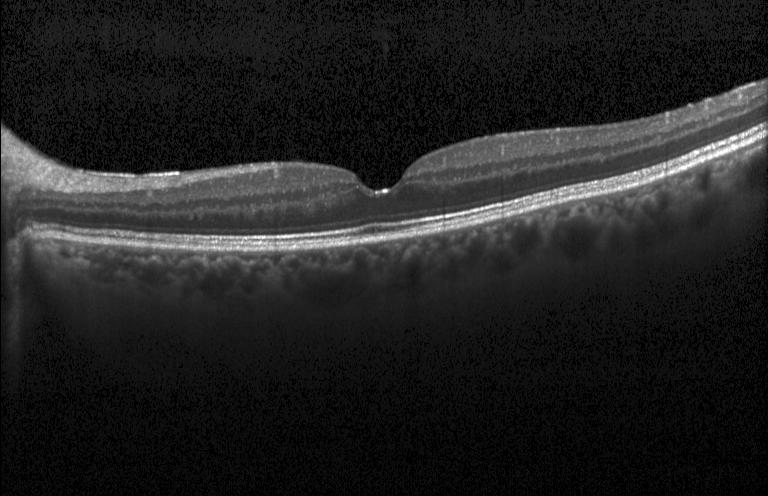

This B-scan demonstrates no evidence of choroidal neovascularization, diabetic macular edema, or drusen.